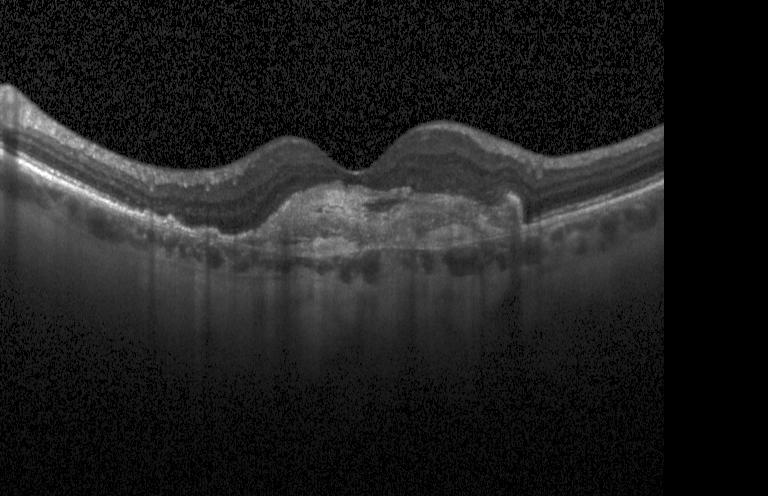

Macular OCT: choroidal neovascularization (CNV).